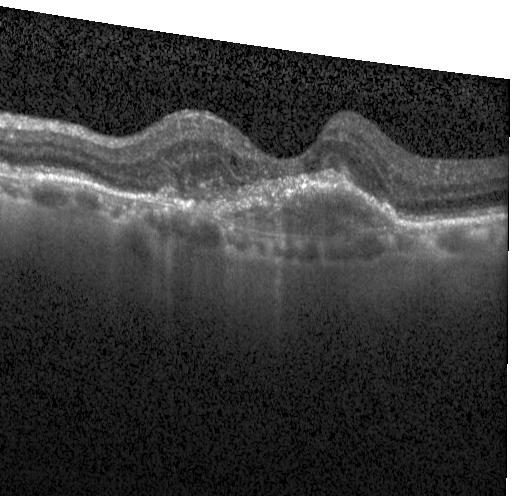 Dx: CNV.